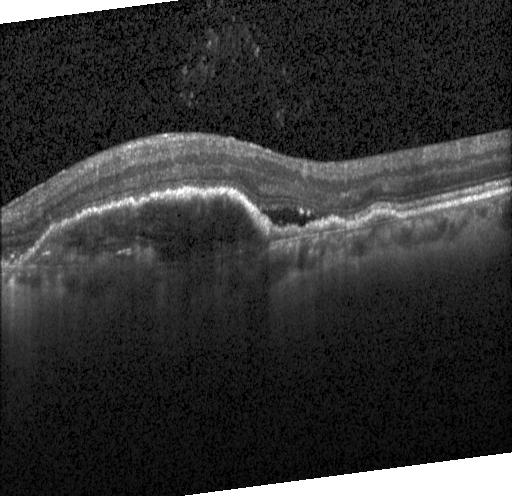
Macular OCT: a choroidal neovascular membrane.